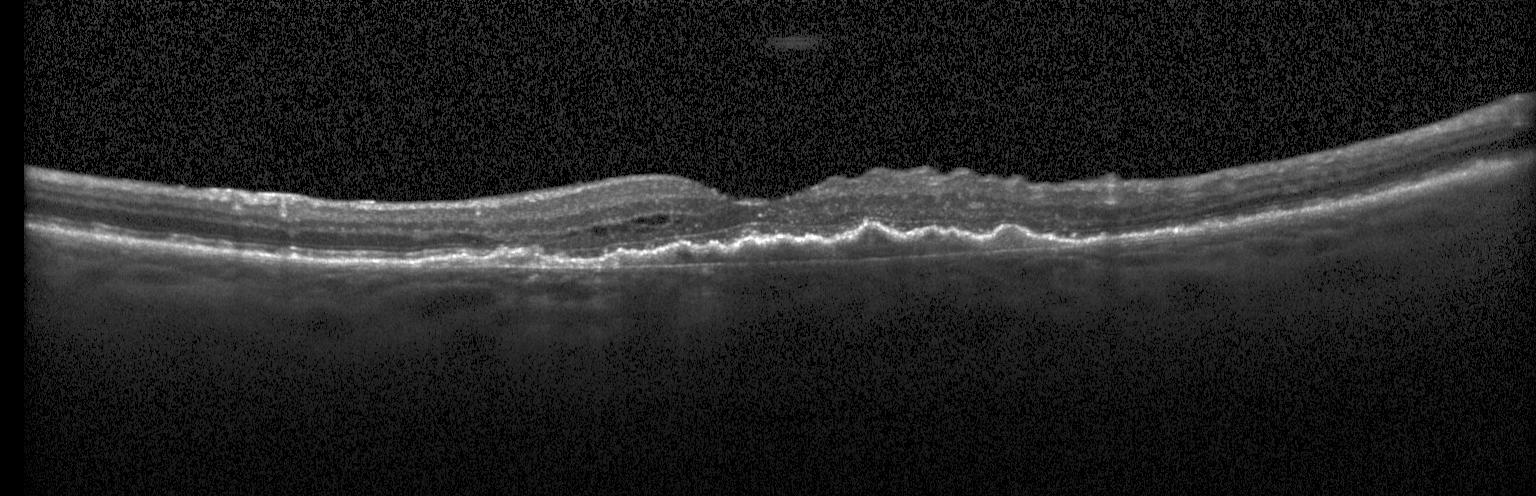 Diagnosis: choroidal neovascularization.